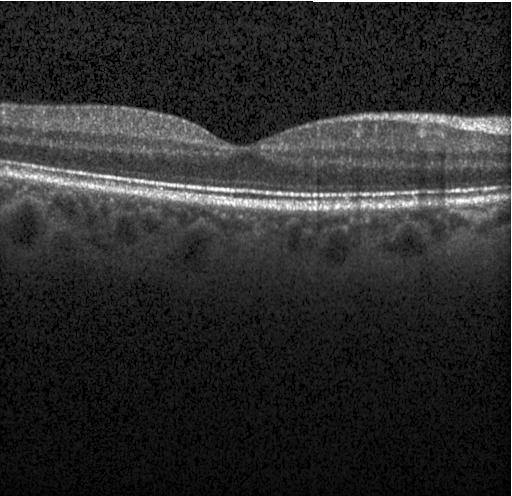
Retinal OCT cross-section, SD-OCT, fovea-centered, acquired on a Heidelberg Spectralis
This B-scan demonstrates no choroidal neovascularization, diabetic macular edema, or drusen.